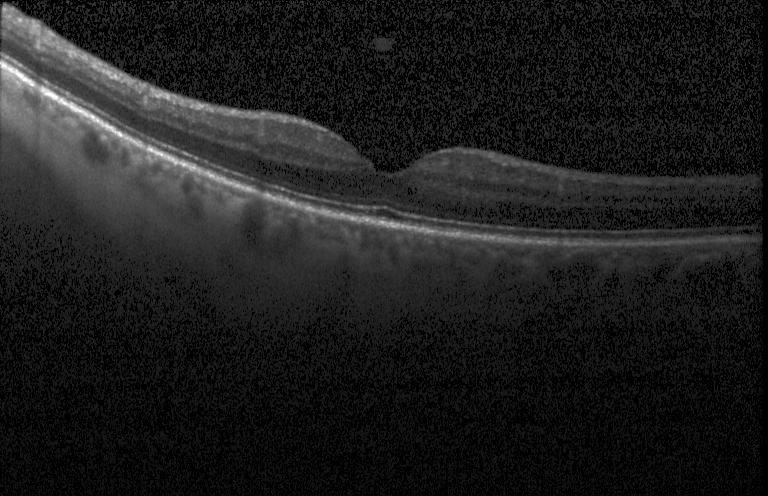

Spectral-domain optical coherence tomography; OCT B-scan.
Diagnosis: no evidence of CNV, DME, or drusen.